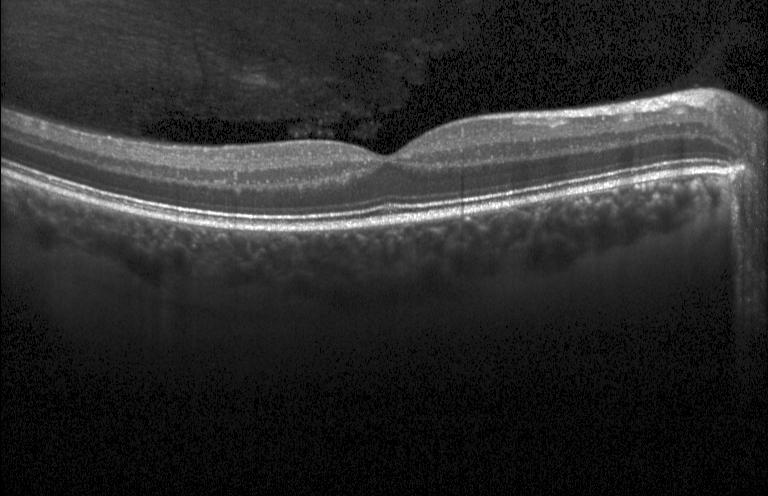

OCT B-scan, Heidelberg Spectralis OCT system.
Impression: no CNV, no DME, and no drusen.